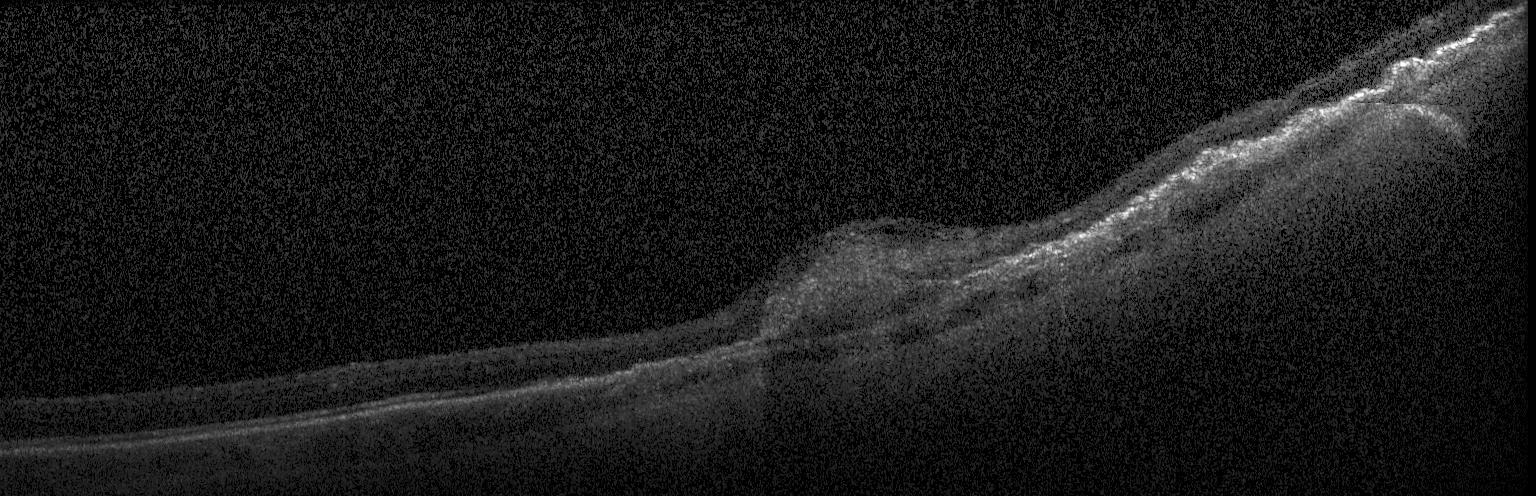

Spectral-domain optical coherence tomography, retinal OCT B-scan.
Finding: choroidal neovascularization (CNV).